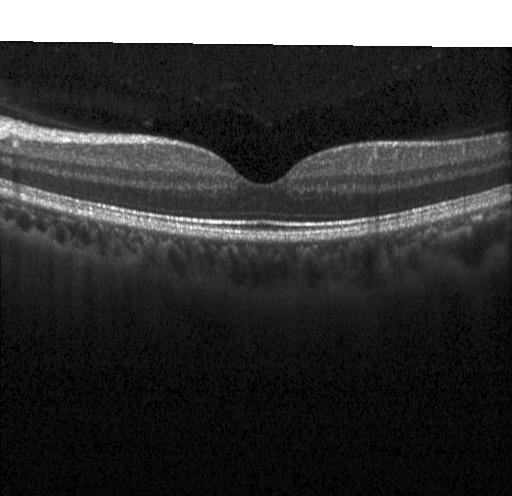

Retinal OCT B-scan; through the macula.
OCT finding: no evidence of choroidal neovascularization, diabetic macular edema, or drusen.